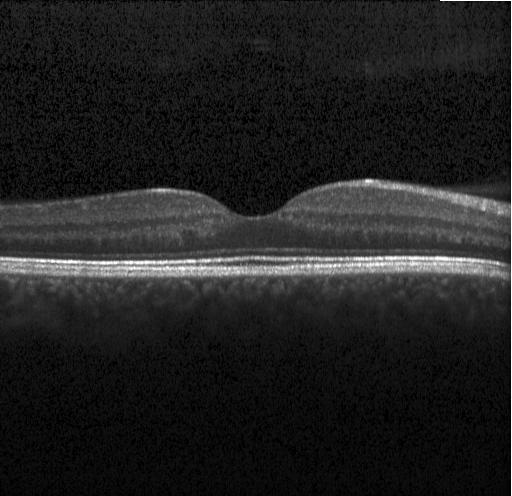
Macular OCT: no evidence of CNV, DME, or drusen.